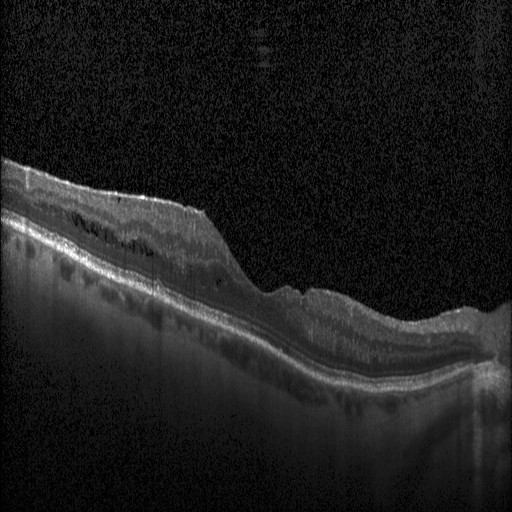 Assessment: diabetic macular edema.